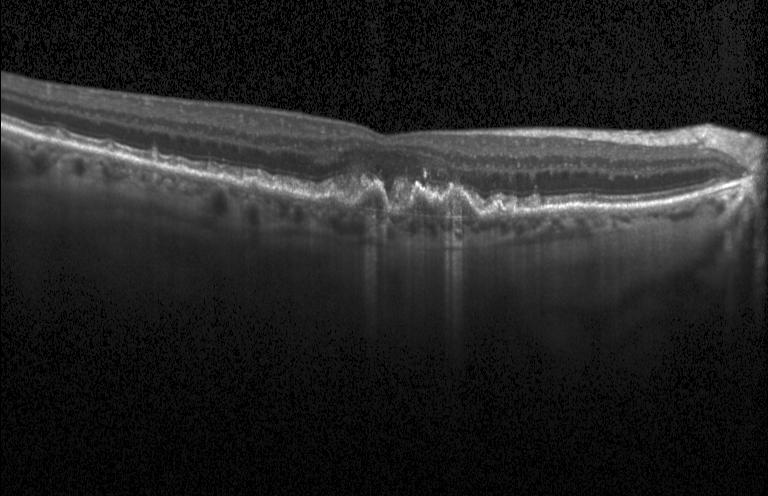 Heidelberg Spectralis. Horizontal scan through the fovea. Retinal OCT B-scan — The scan shows a choroidal neovascular membrane.